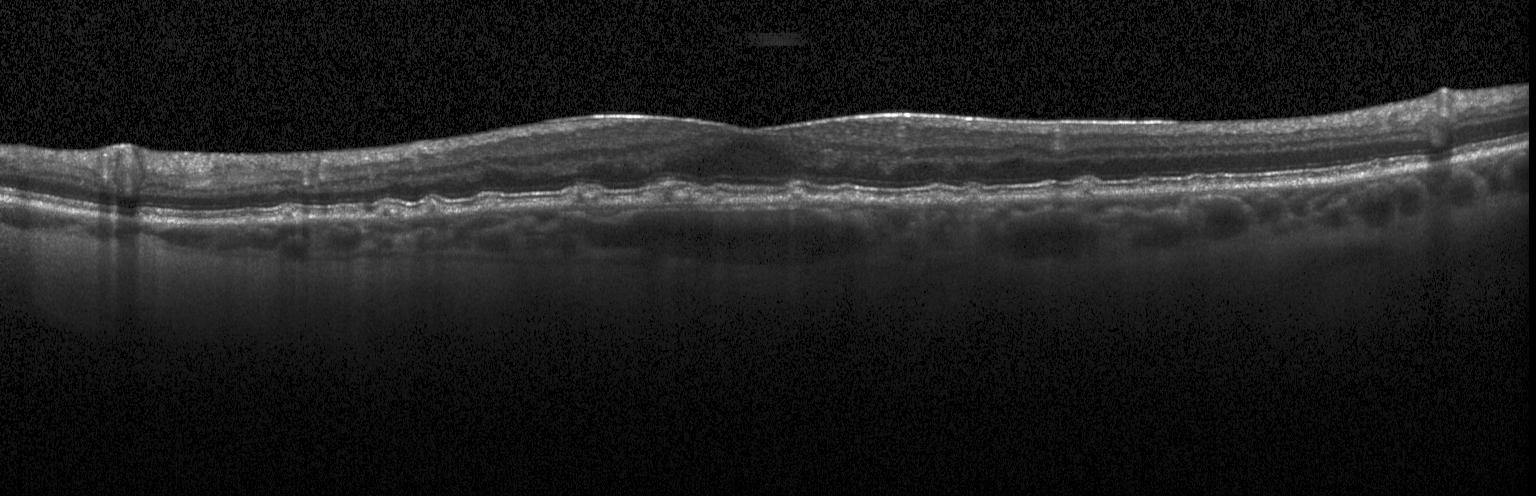
Acquired on a Heidelberg Spectralis. OCT B-scan. Centered on the fovea — Diagnosis: sub-RPE drusenoid deposits.